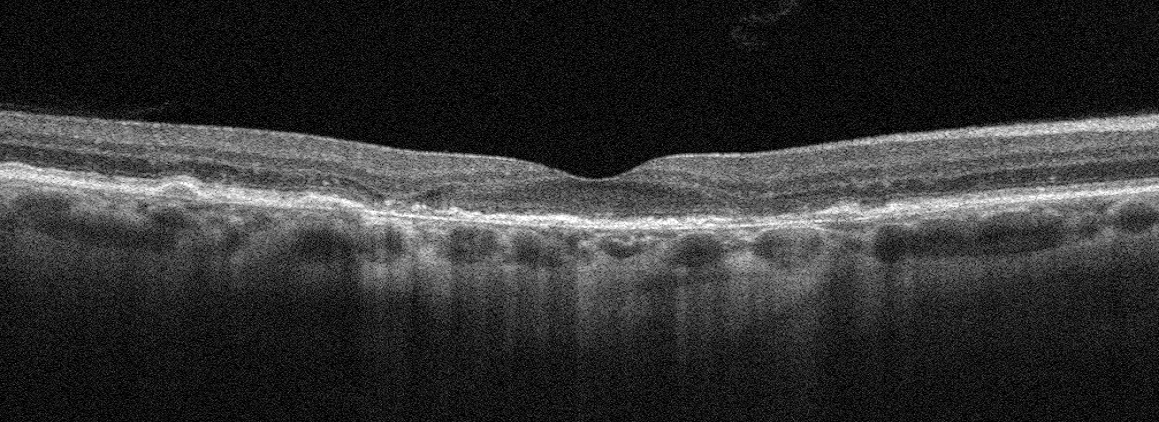

Optical coherence tomography scan. Right eye
OCT finding: age-related macular degeneration (AMD).